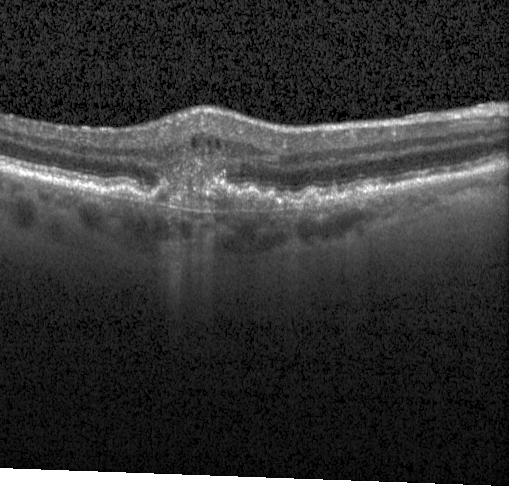
Finding: a choroidal neovascular membrane.